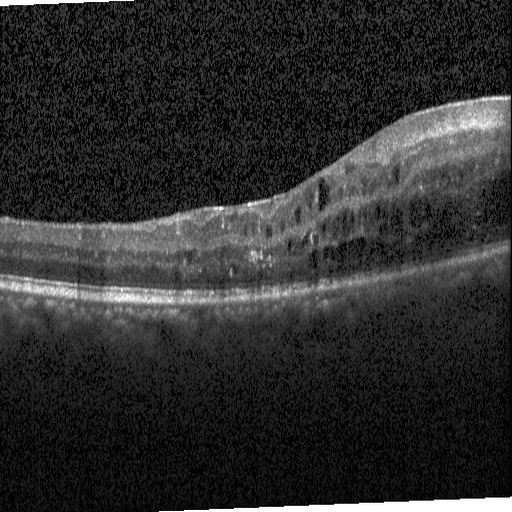 Assessment: diabetic macular edema.